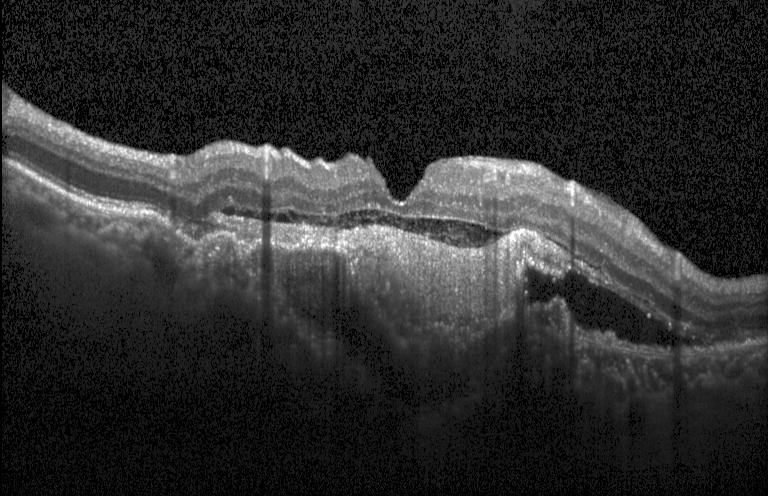

OCT B-scan showing CNV.